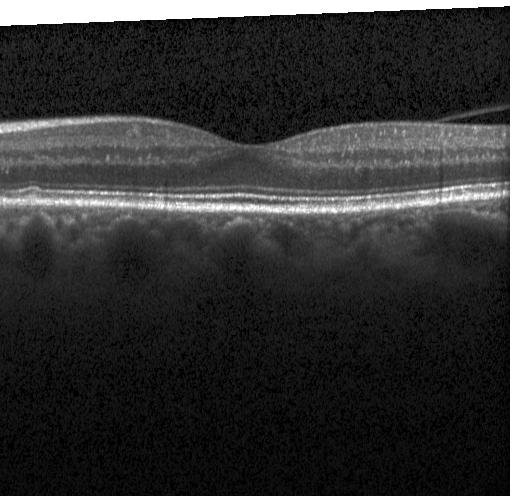 Finding: drusen.